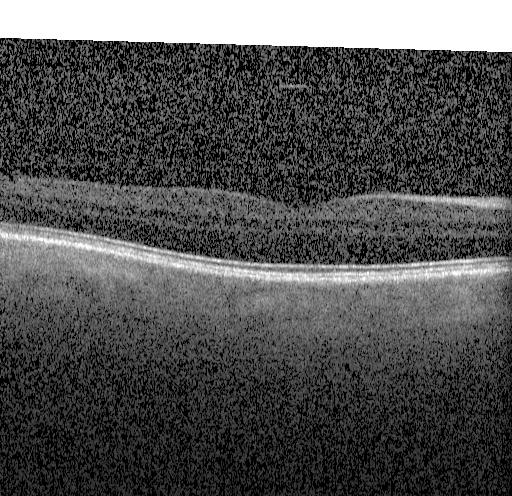
The scan shows no CNV, DME, or drusen.